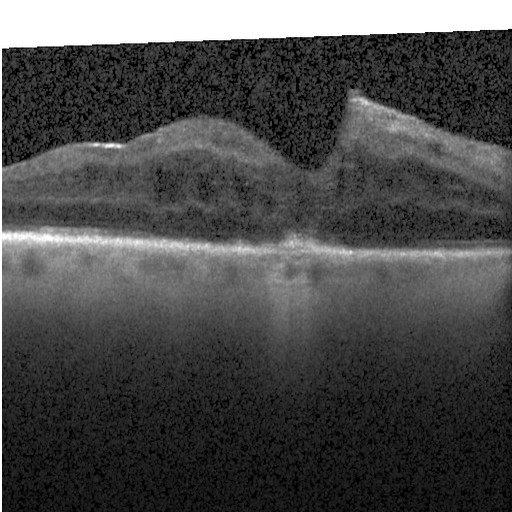

Diagnosis: diabetic macular edema (DME).